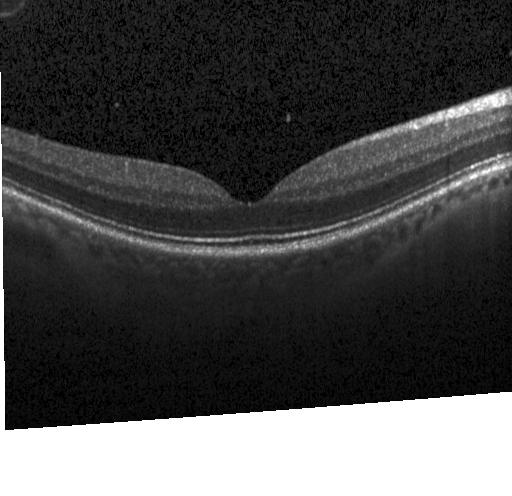 Assessment: neither CNV, DME, nor drusen.